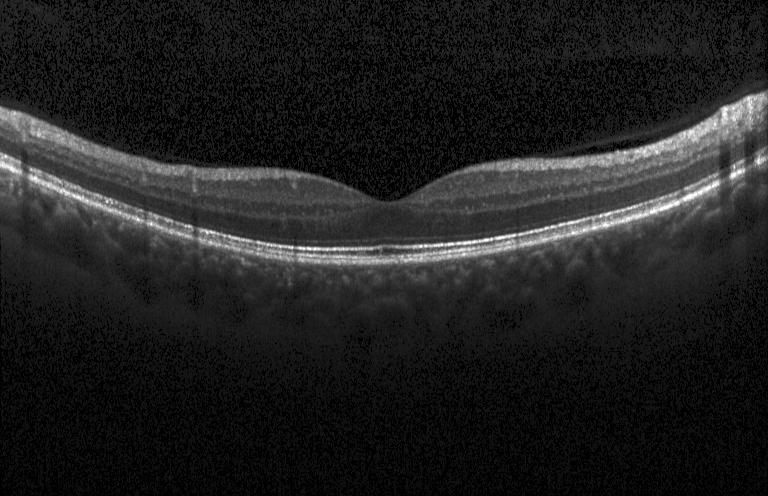 Retinal OCT cross-section, Heidelberg Spectralis OCT system, macular scan
Impression: no choroidal neovascularization, no diabetic macular edema, and no drusen.